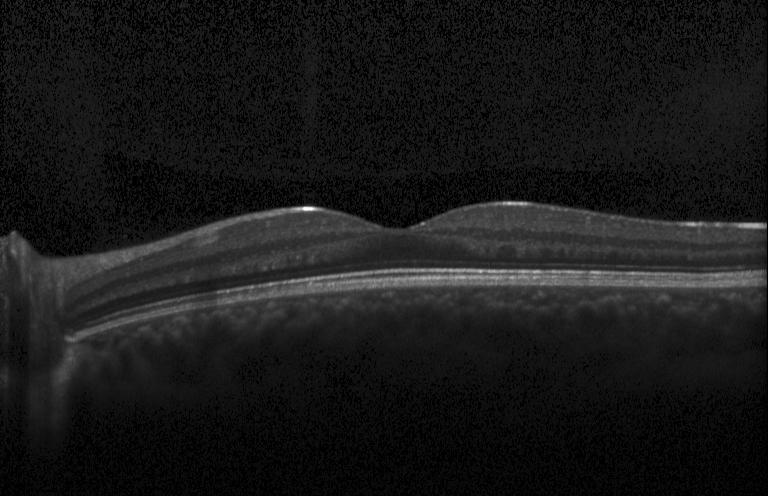
OCT B-scan showing no CNV, no DME, and no drusen.